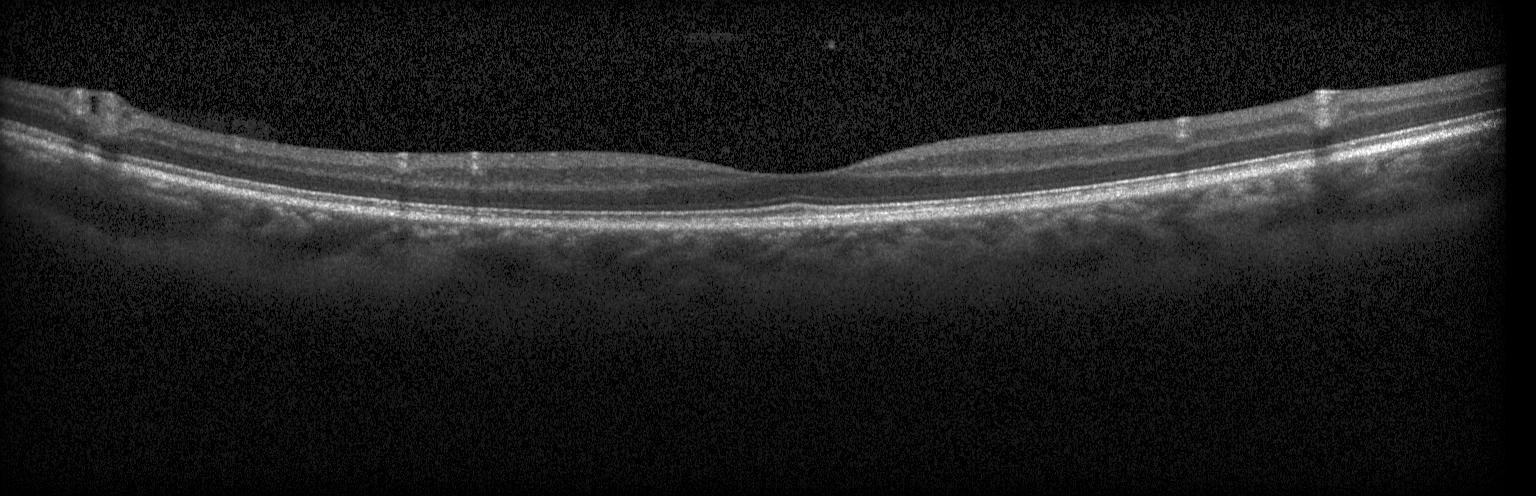 Impression: no evidence of CNV, DME, or drusen.